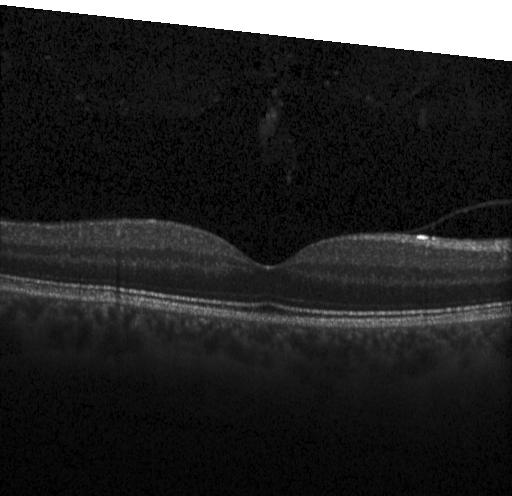 OCT finding: no choroidal neovascularization, diabetic macular edema, or drusen.